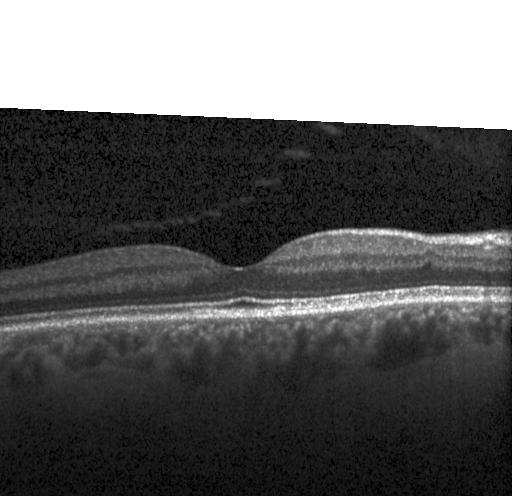 Optical coherence tomography B-scan
Finding: no choroidal neovascularization, diabetic macular edema, or drusen.